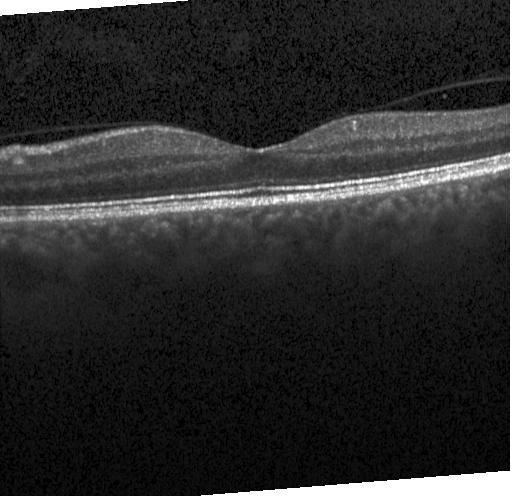

OCT B-scan.
Macular OCT: no choroidal neovascularization, diabetic macular edema, or drusen.